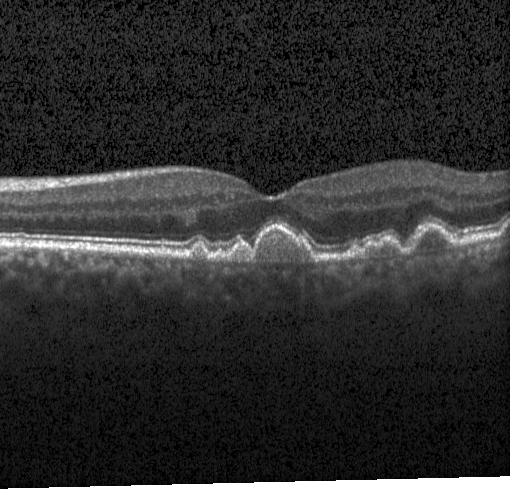
The scan shows sub-RPE drusenoid deposits.